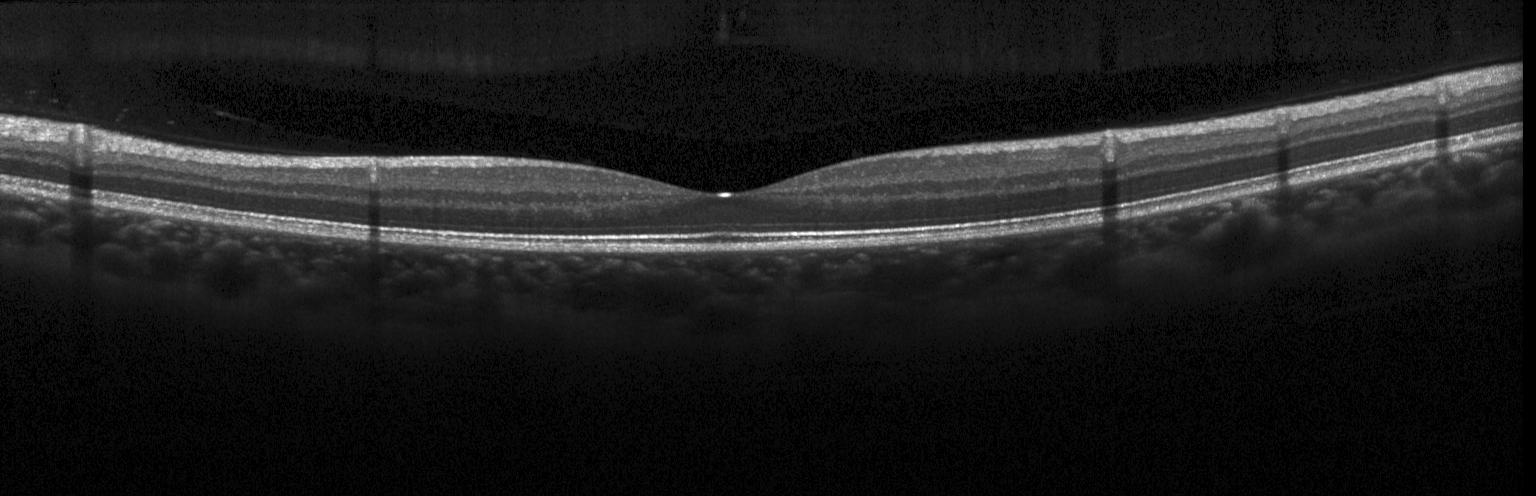
OCT B-scan showing no CNV, no DME, and no drusen.